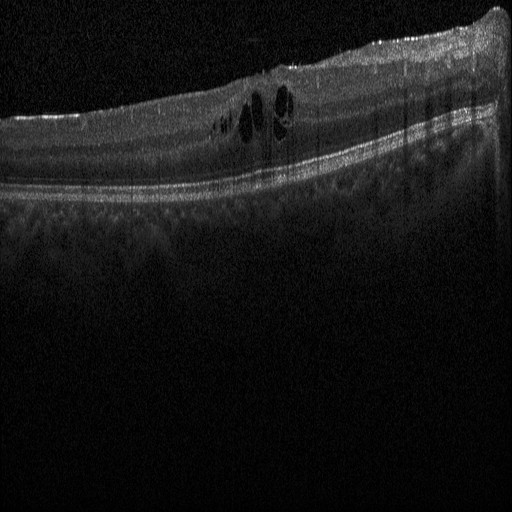

Finding: diabetic macular edema.